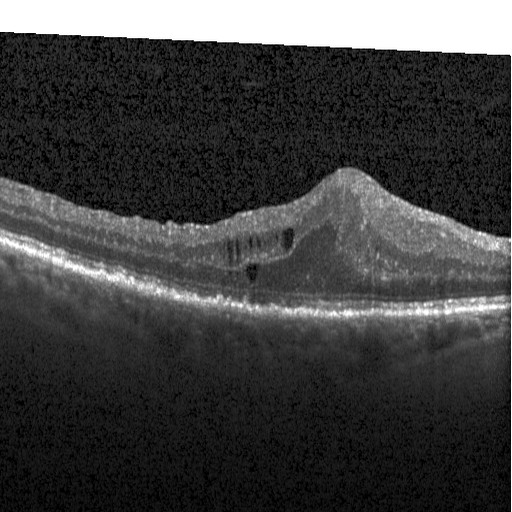
OCT B-scan. Diagnosis: diabetic macular edema.